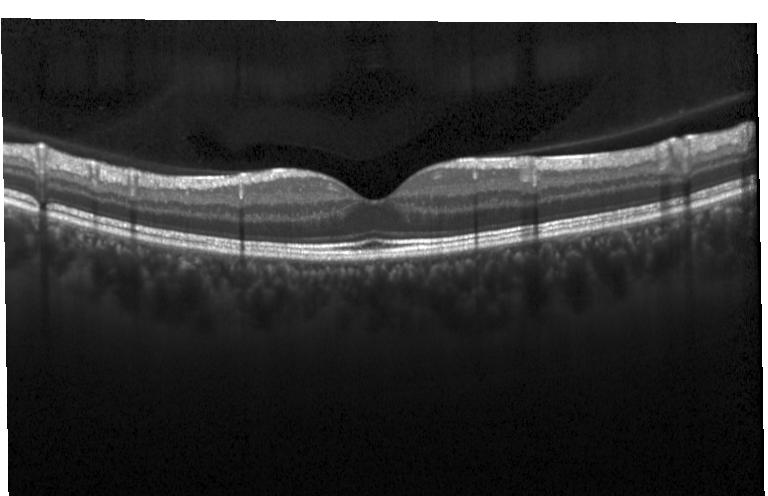
Diagnosis: no evidence of choroidal neovascularization, diabetic macular edema, or drusen.